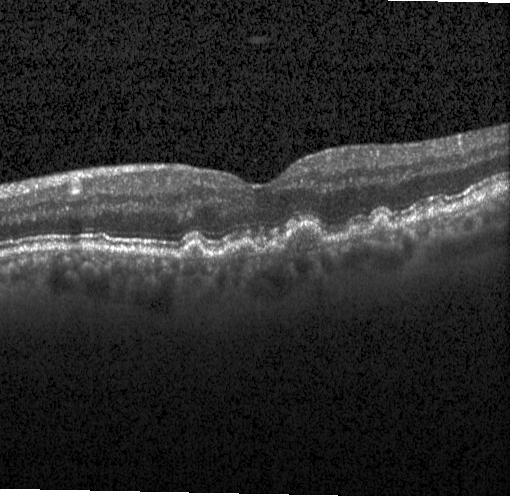

Macular scan. Spectral-domain optical coherence tomography. Optical coherence tomography B-scan — Macular OCT: sub-RPE drusenoid deposits.